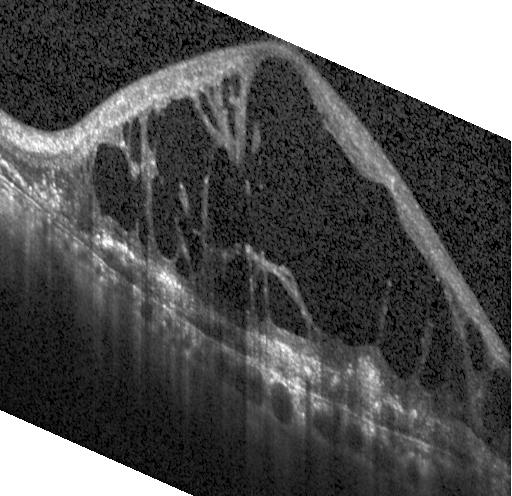 CNV.